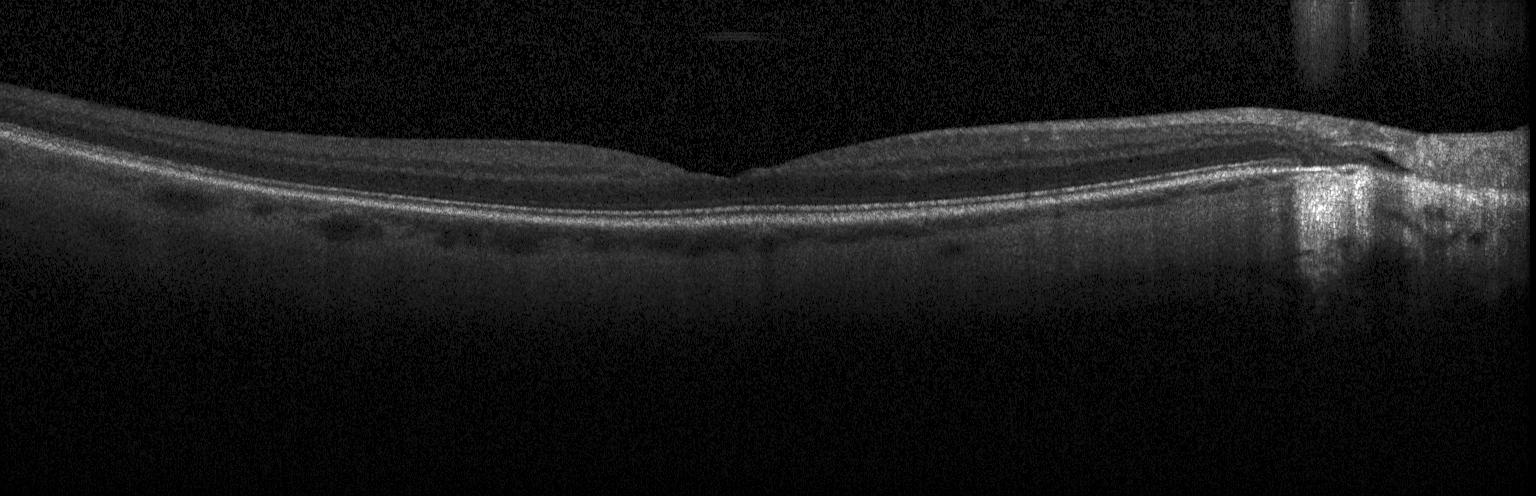
Finding: no choroidal neovascularization, no diabetic macular edema, and no drusen.